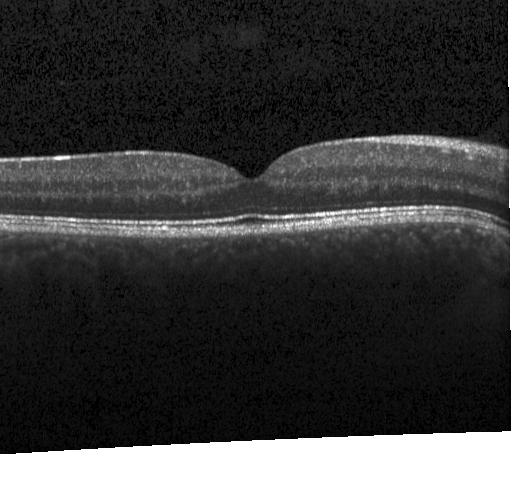
This B-scan demonstrates neither choroidal neovascularization, diabetic macular edema, nor drusen.